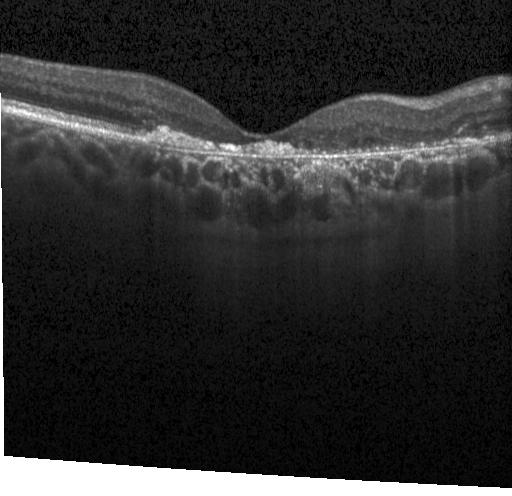
Macular OCT demonstrating choroidal neovascularization.